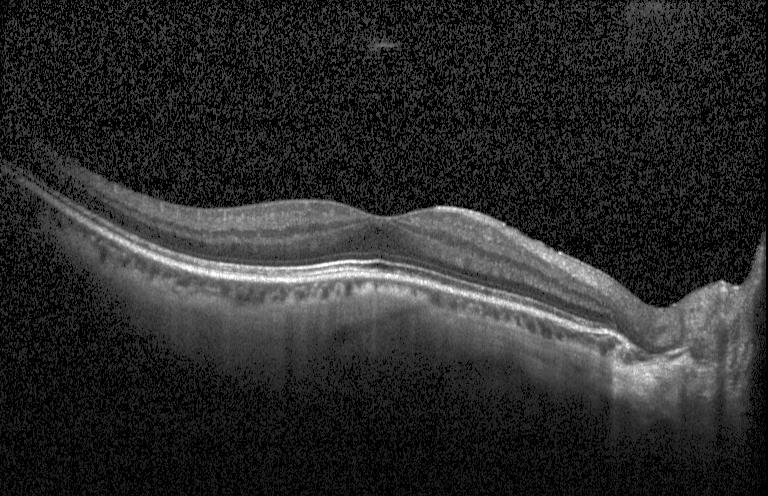
OCT B-scan
Neither CNV, DME, nor drusen.